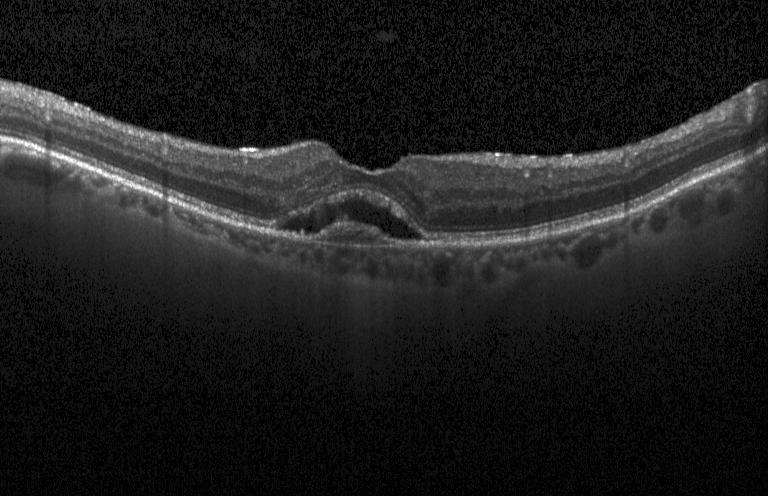
OCT finding: choroidal neovascularization.